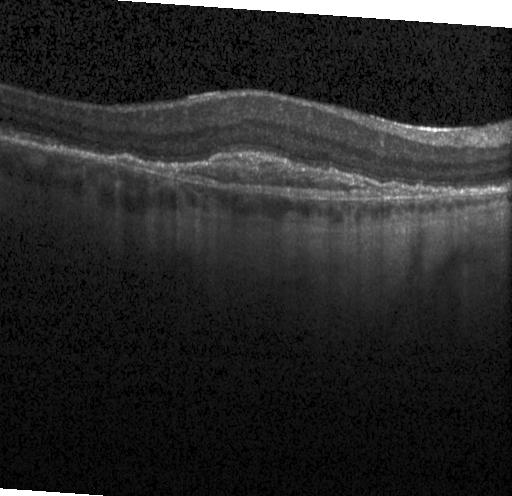

The scan shows choroidal neovascularization (CNV).